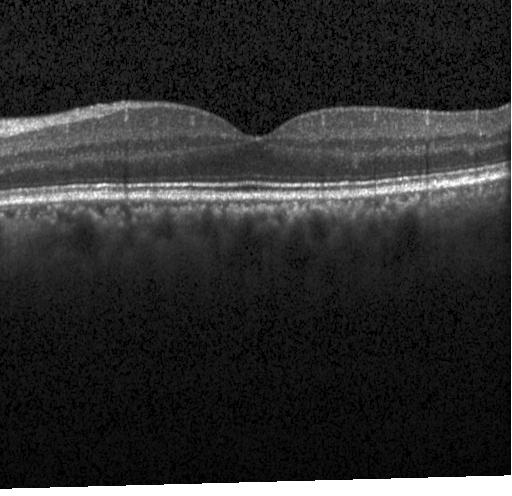 SD-OCT; retinal OCT cross-section — Finding: neither choroidal neovascularization, diabetic macular edema, nor drusen.